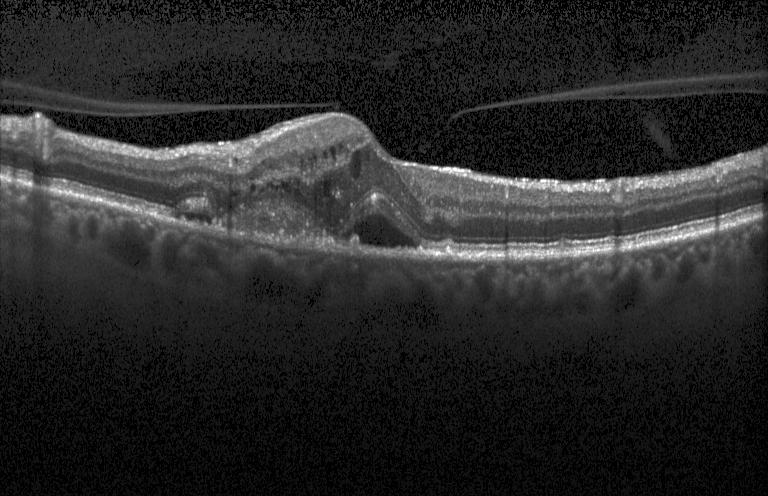

OCT scan showing a choroidal neovascular membrane.